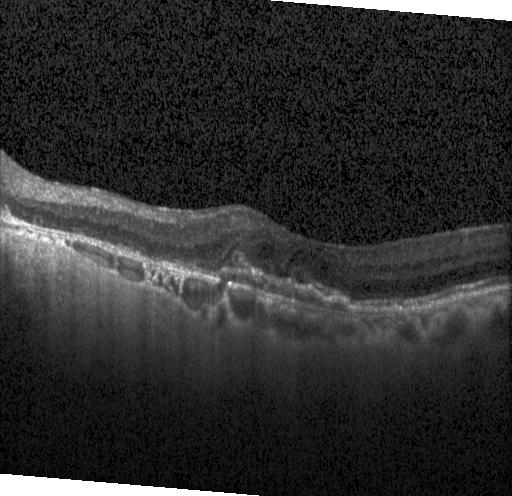 Spectral-domain optical coherence tomography; OCT line scan; macular scan
Diagnosis: CNV.